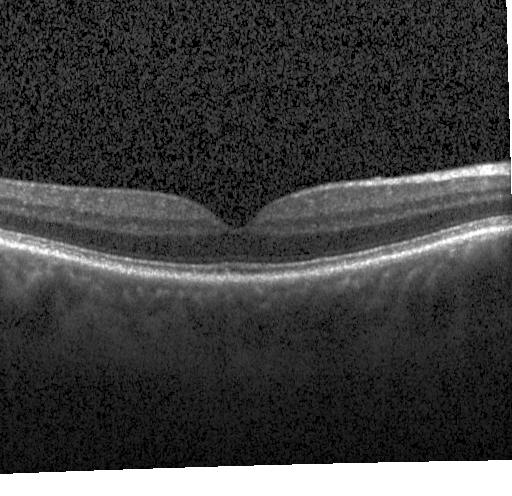
Through the macula, spectral-domain optical coherence tomography, instrument: Heidelberg Spectralis, retinal OCT cross-section
This B-scan demonstrates neither choroidal neovascularization, diabetic macular edema, nor drusen.